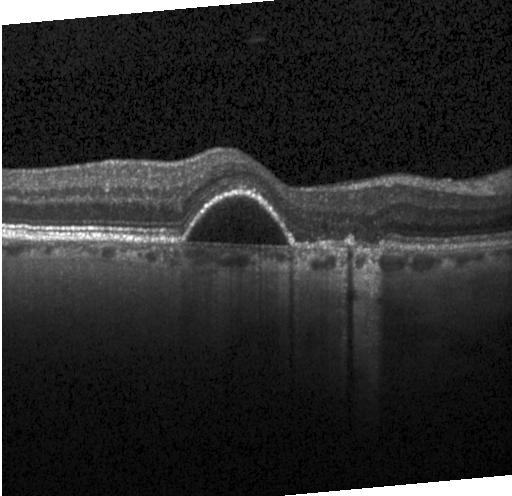
Optical coherence tomography scan.
Assessment: choroidal neovascularization (CNV).